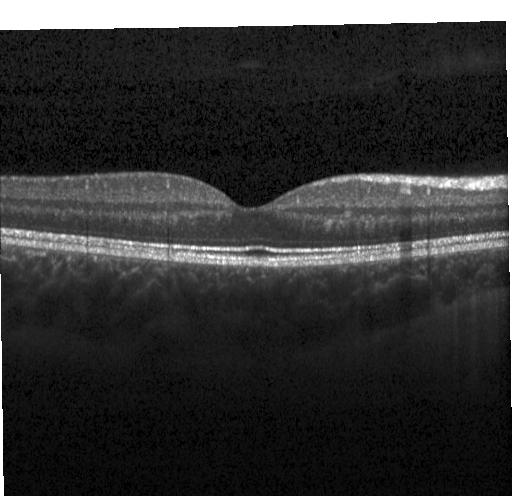
Spectral-domain optical coherence tomography, acquired on a Heidelberg Spectralis, retinal OCT cross-section. The scan shows no choroidal neovascularization, no diabetic macular edema, and no drusen.